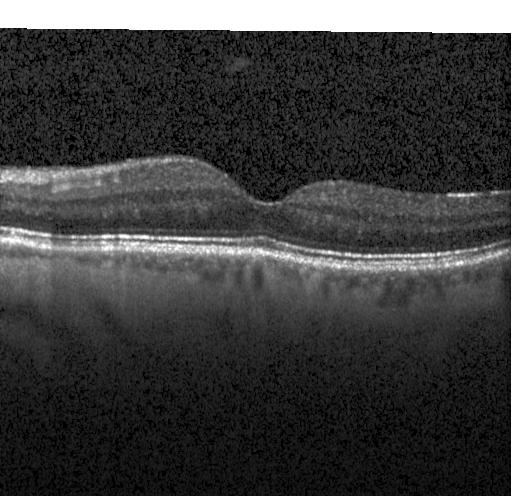 Diagnosis: no evidence of choroidal neovascularization, diabetic macular edema, or drusen.